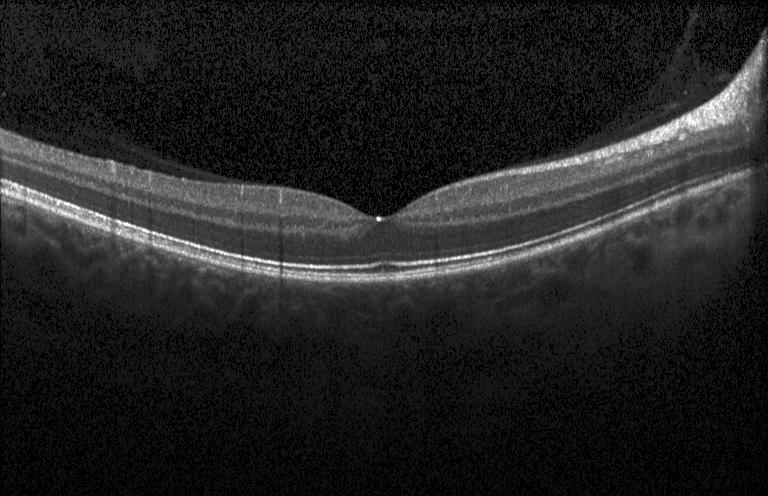 Heidelberg Spectralis OCT system, optical coherence tomography scan, spectral-domain OCT, centered on the fovea — Diagnosis: no choroidal neovascularization, diabetic macular edema, or drusen.